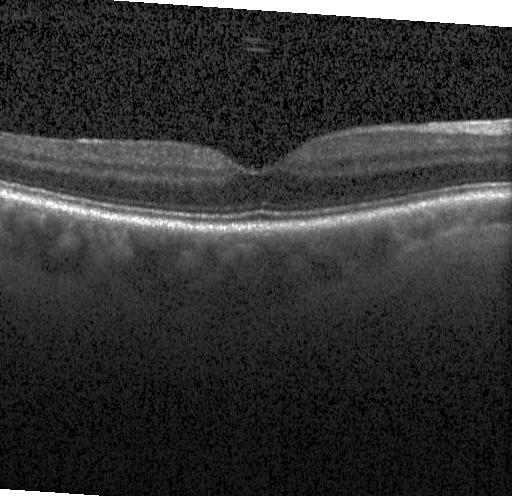

Optical coherence tomography B-scan.
This B-scan demonstrates no choroidal neovascularization, no diabetic macular edema, and no drusen.